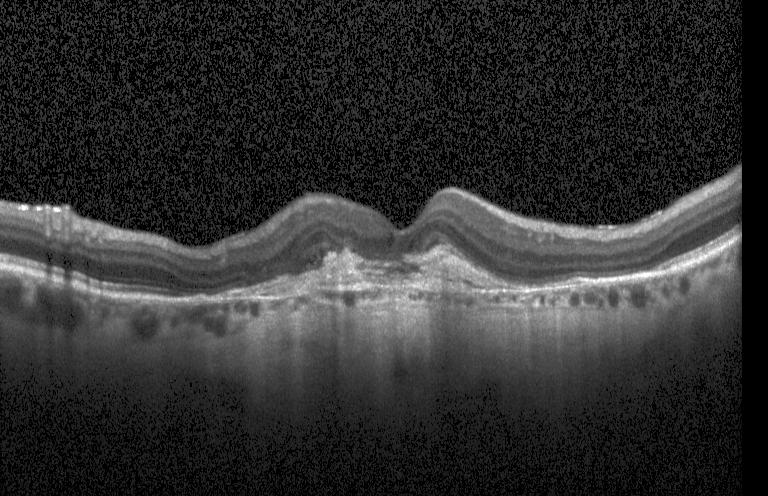 Impression: CNV.